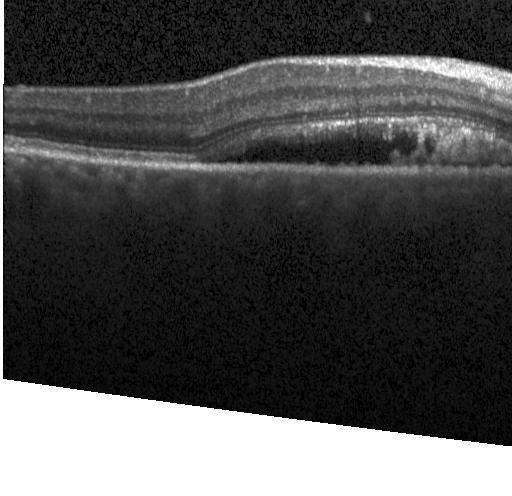 Heidelberg Spectralis; centered on the fovea; OCT B-scan; spectral-domain OCT.
This B-scan demonstrates a choroidal neovascular membrane.